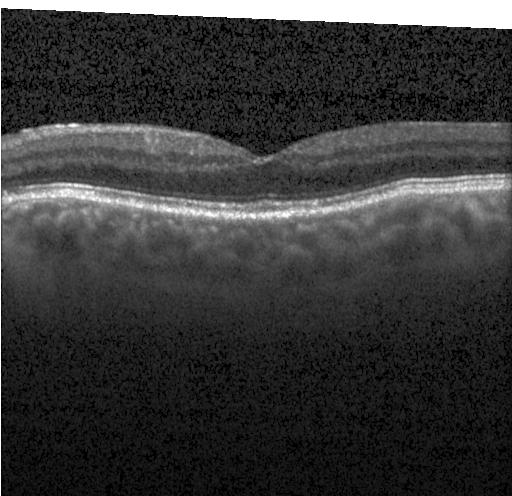

Finding: neither choroidal neovascularization, diabetic macular edema, nor drusen.